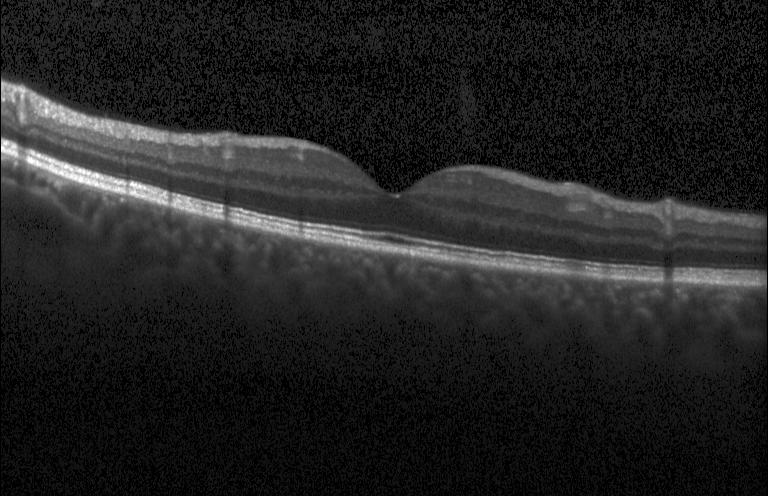
Finding: no choroidal neovascularization, no diabetic macular edema, and no drusen.